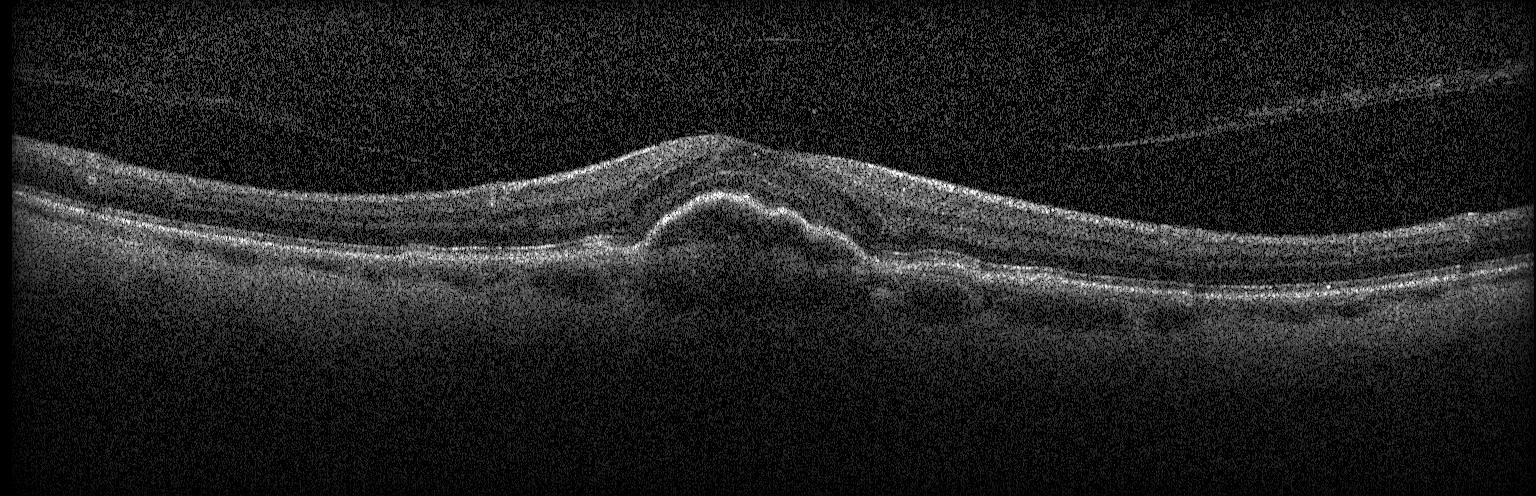 OCT B-scan showing a choroidal neovascular membrane.